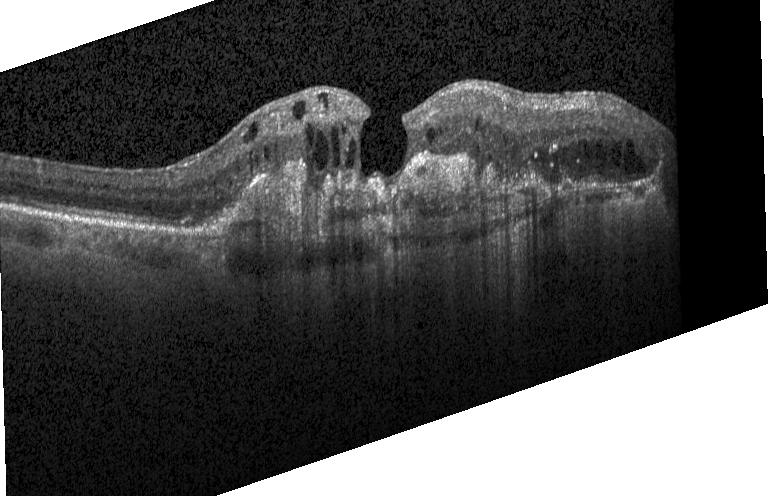
OCT B-scan. The scan shows choroidal neovascularization.